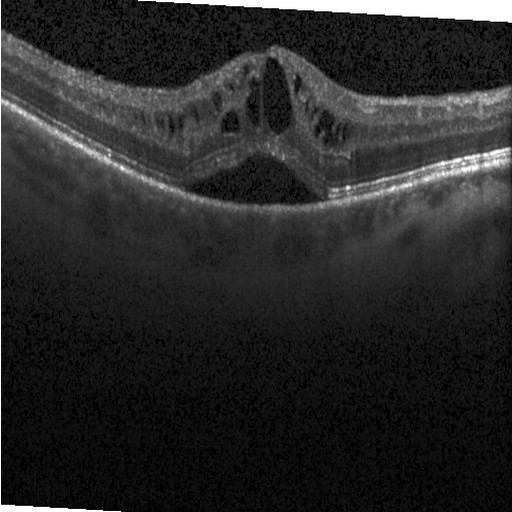 Heidelberg Spectralis · centered on the fovea · optical coherence tomography scan.
Diagnosis: DME.